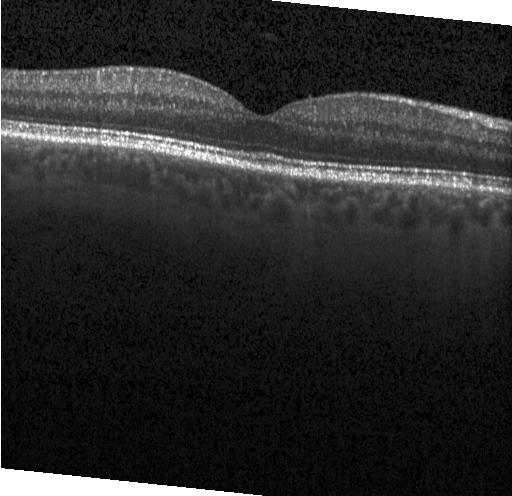 Neither CNV, DME, nor drusen.